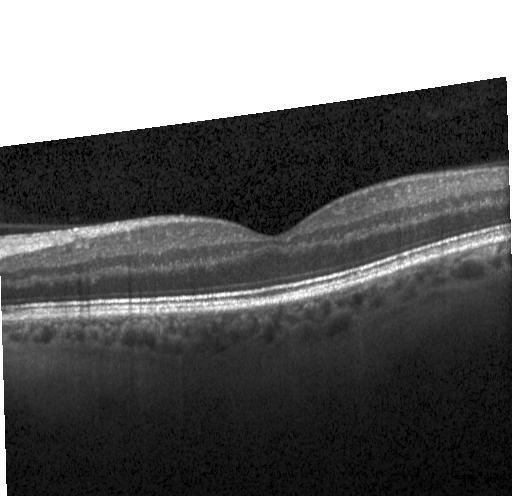 Assessment: no evidence of choroidal neovascularization, diabetic macular edema, or drusen.